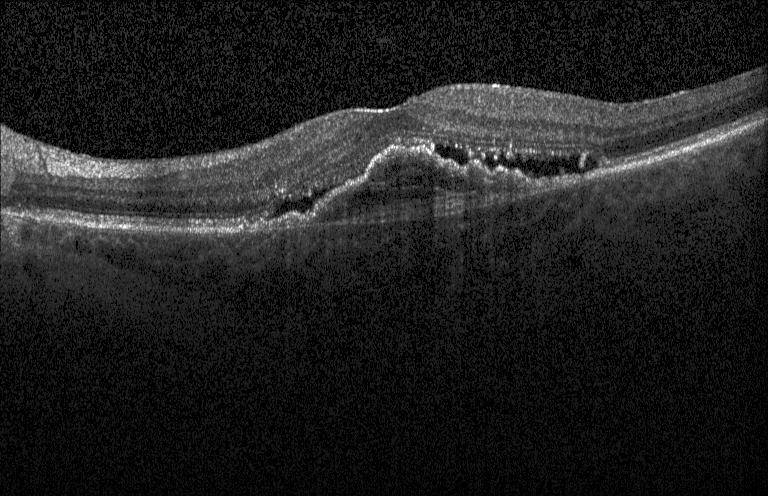 Diagnosis: a choroidal neovascular membrane.